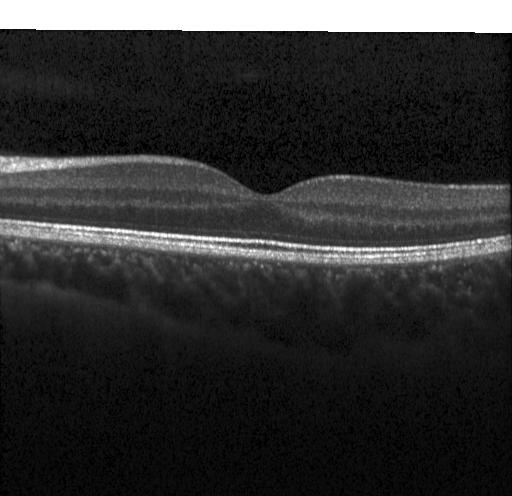
OCT B-scan — Macular OCT: no CNV, DME, or drusen.